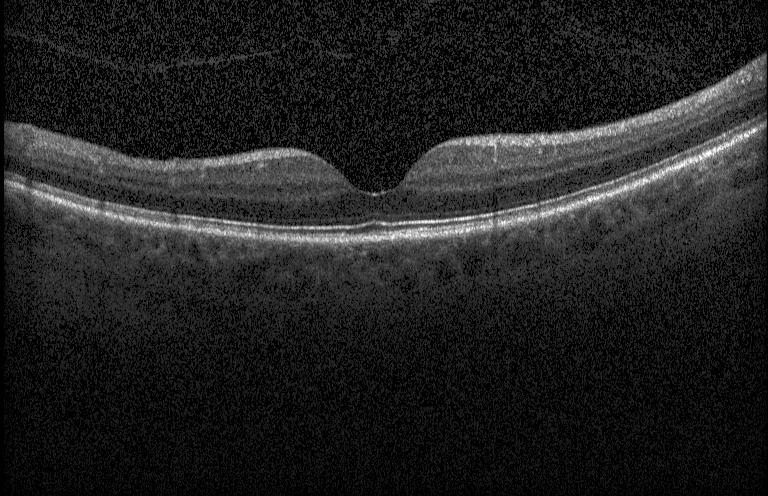
Optical coherence tomography B-scan · acquired on a Heidelberg Spectralis. The scan shows neither choroidal neovascularization, diabetic macular edema, nor drusen.